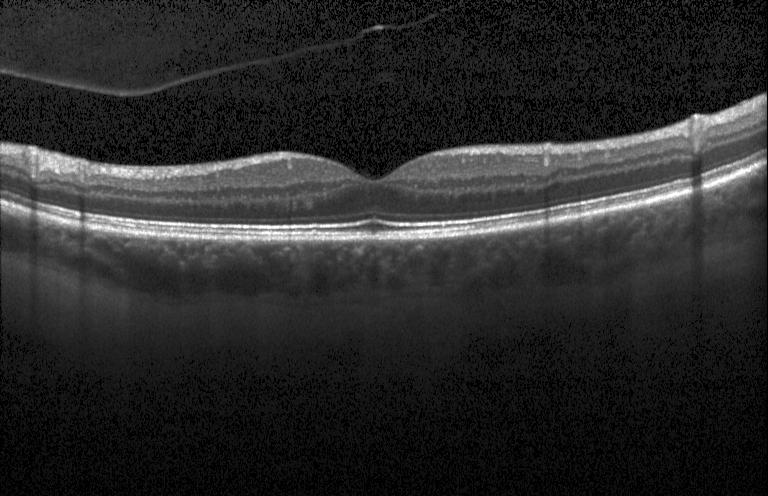

OCT scan showing neither choroidal neovascularization, diabetic macular edema, nor drusen.